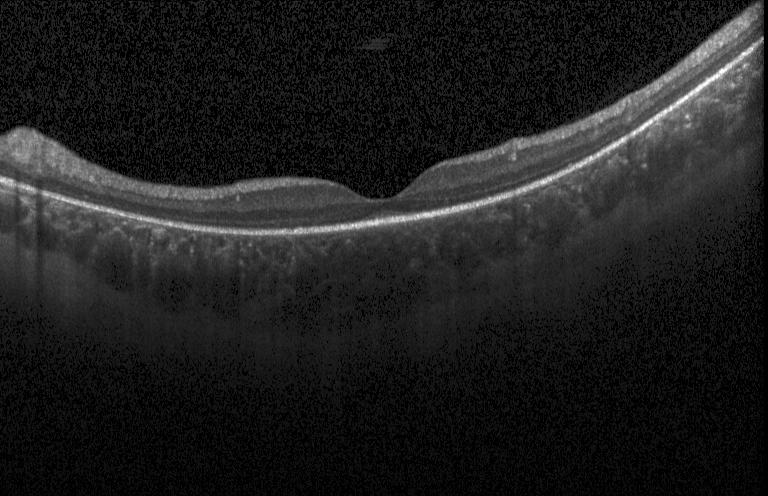
The scan shows no evidence of choroidal neovascularization, diabetic macular edema, or drusen.